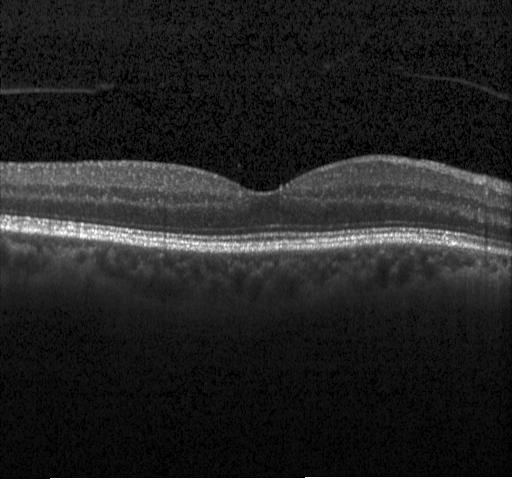
Retinal OCT cross-section; macular scan; instrument: Heidelberg Spectralis.
Impression: no choroidal neovascularization, no diabetic macular edema, and no drusen.